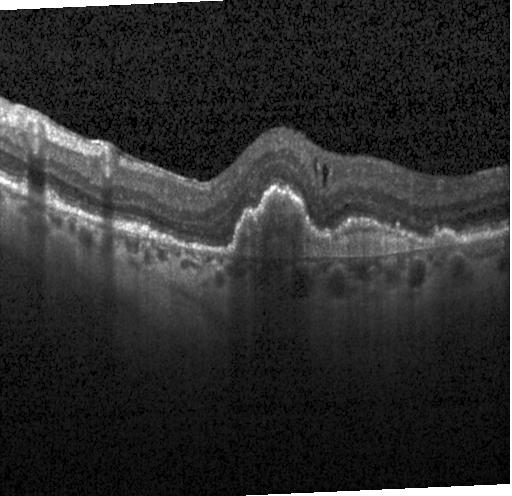
Instrument: Heidelberg Spectralis, retinal OCT cross-section
Impression: a choroidal neovascular membrane.